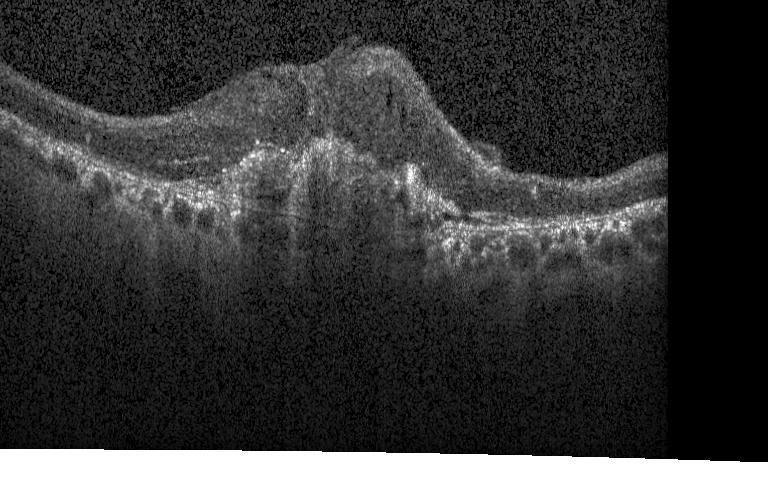
Heidelberg Spectralis · centered on the fovea · retinal OCT cross-section · SD-OCT
Impression: a choroidal neovascular membrane.